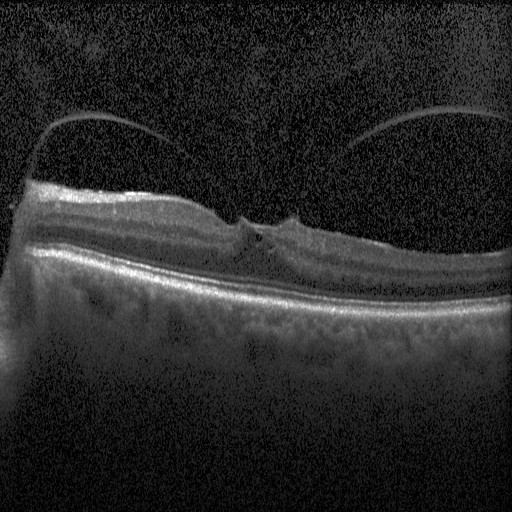 Instrument: Heidelberg Spectralis. Centered on the fovea. OCT line scan. Spectral-domain OCT.
Assessment: DME.